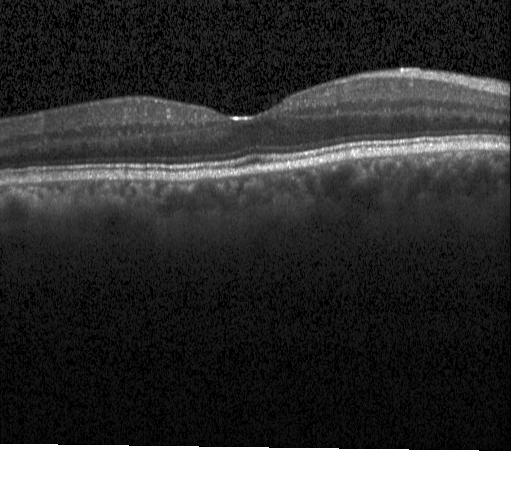
Instrument: Heidelberg Spectralis. Fovea-centered. Spectral-domain optical coherence tomography. Optical coherence tomography B-scan.
No choroidal neovascularization, diabetic macular edema, or drusen.